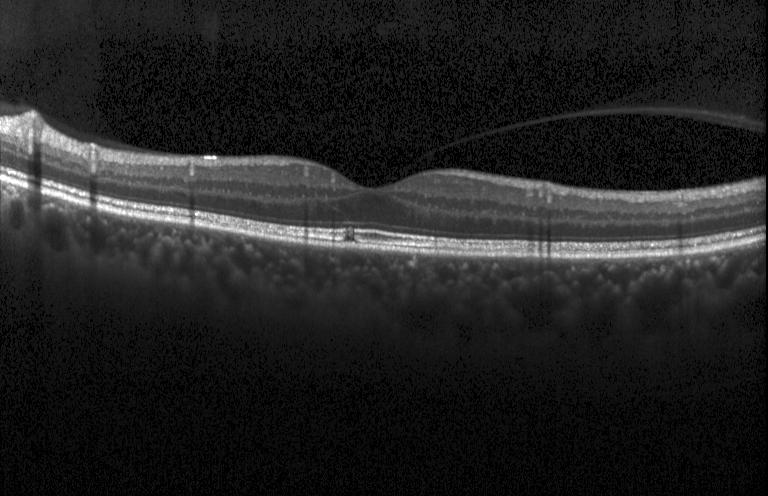
Spectral-domain OCT, retinal OCT cross-section, Heidelberg Spectralis OCT system
The scan shows neither choroidal neovascularization, diabetic macular edema, nor drusen.